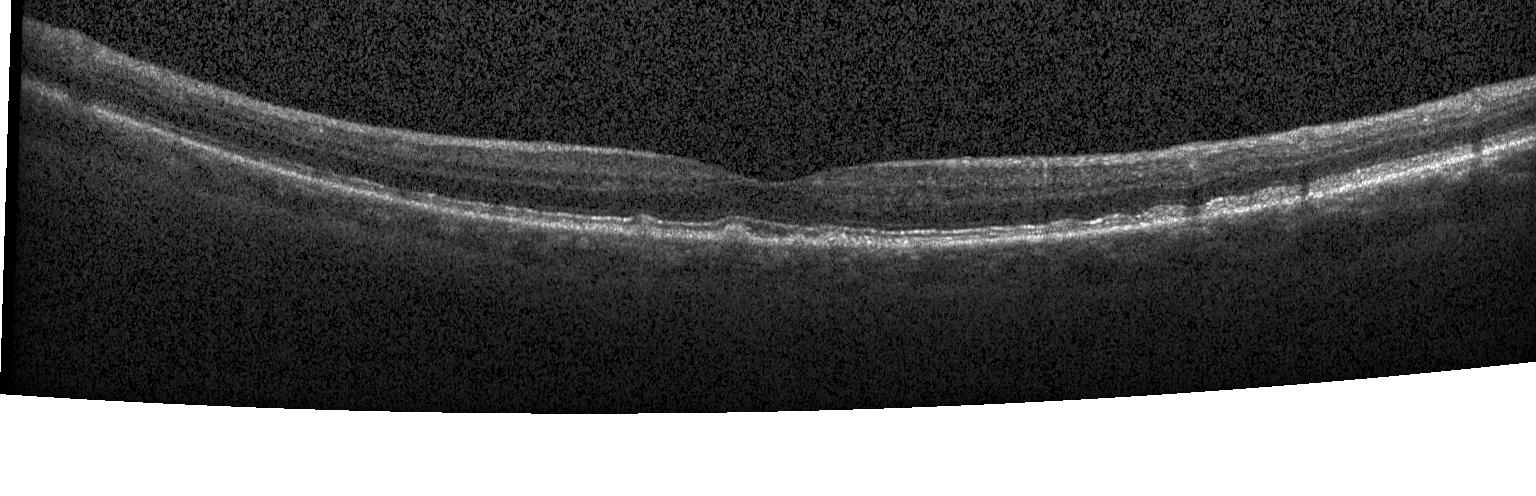

Spectral-domain OCT · OCT line scan · macular scan.
Diagnosis: sub-RPE drusenoid deposits.